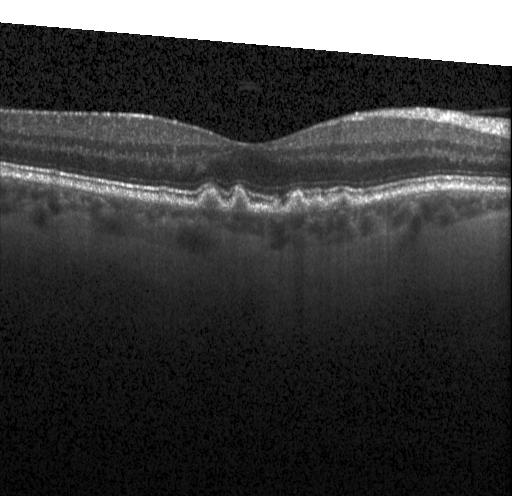

Horizontal scan through the fovea, Heidelberg Spectralis OCT system, OCT B-scan.
Impression: drusen.